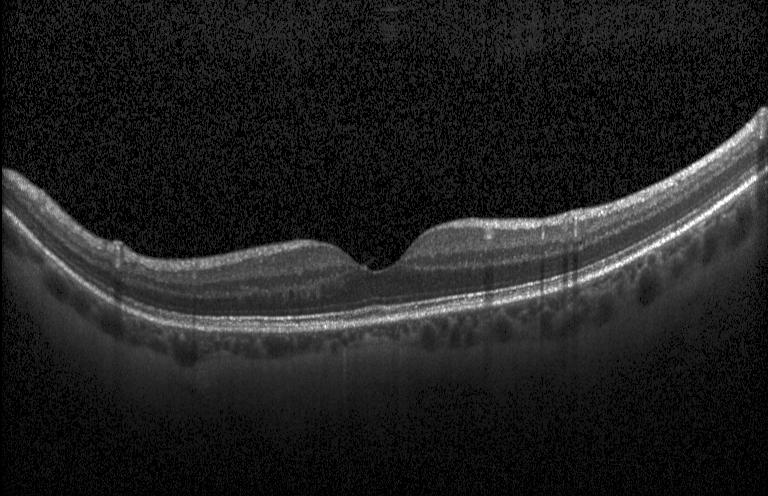 Heidelberg Spectralis OCT system · horizontal scan through the fovea · OCT line scan · SD-OCT
Diagnosis: no choroidal neovascularization, diabetic macular edema, or drusen.